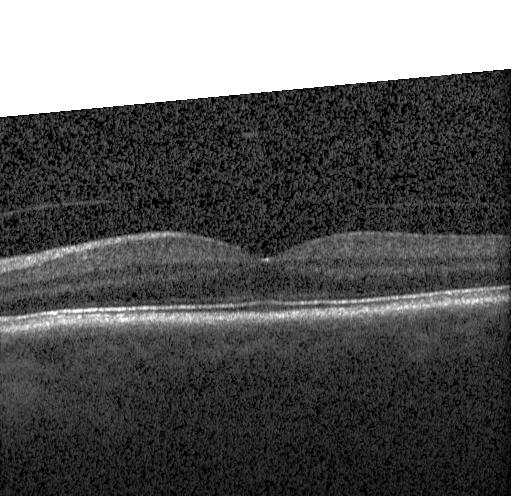
Heidelberg Spectralis; OCT line scan; through the macula; spectral-domain optical coherence tomography
This B-scan demonstrates no CNV, DME, or drusen.